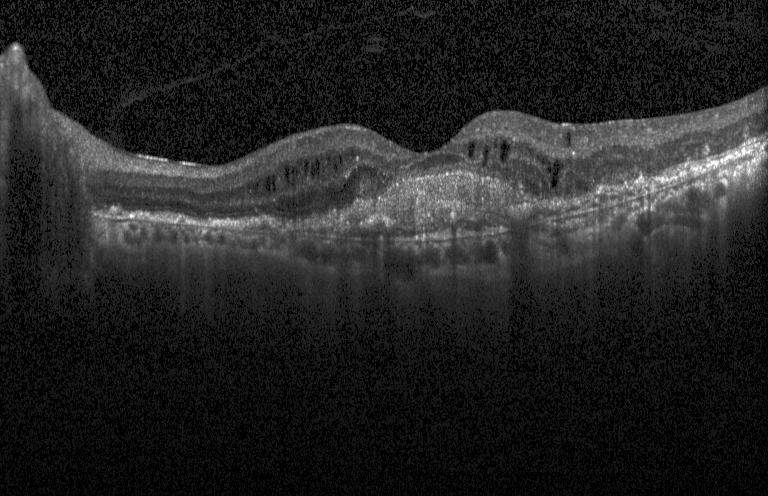 Spectral-domain OCT B-scan: choroidal neovascularization (CNV).